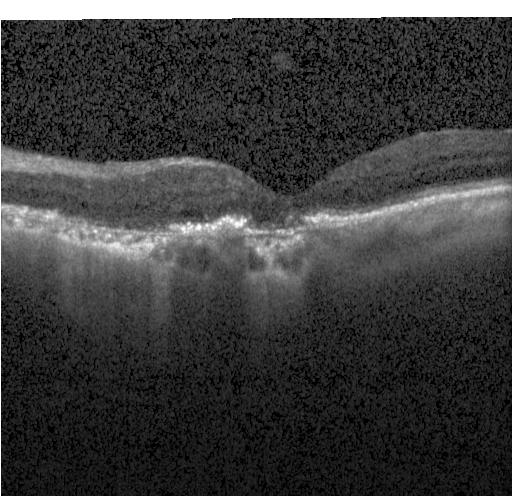
SD-OCT. OCT B-scan
Macular OCT: choroidal neovascularization.